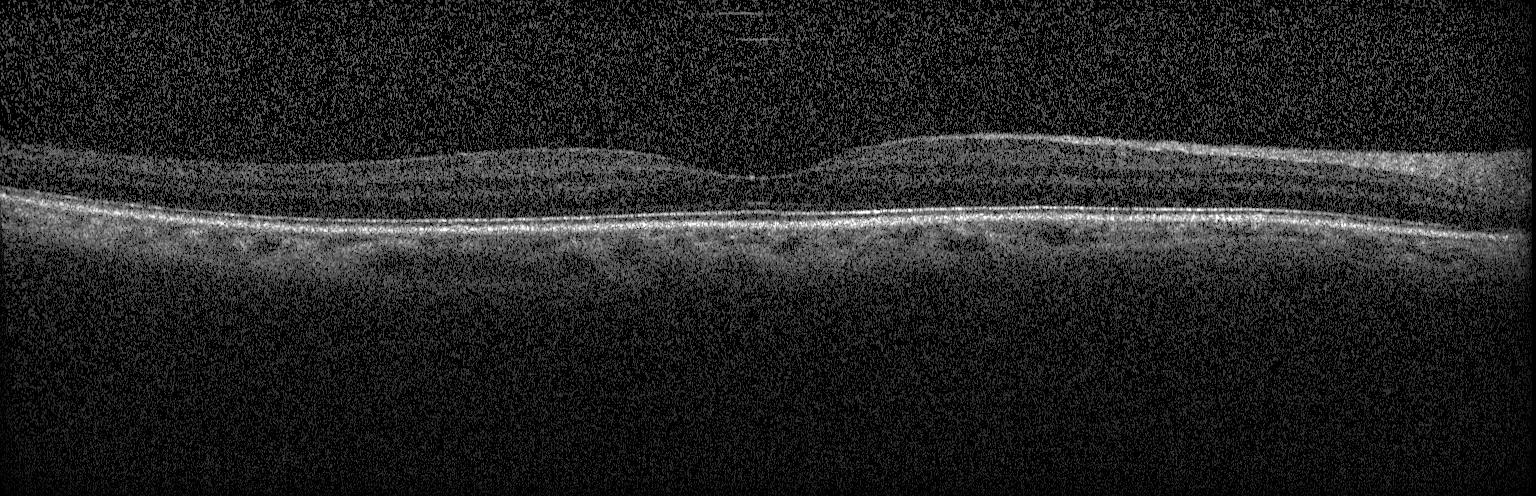 OCT line scan; Heidelberg Spectralis. Dx: no evidence of choroidal neovascularization, diabetic macular edema, or drusen.